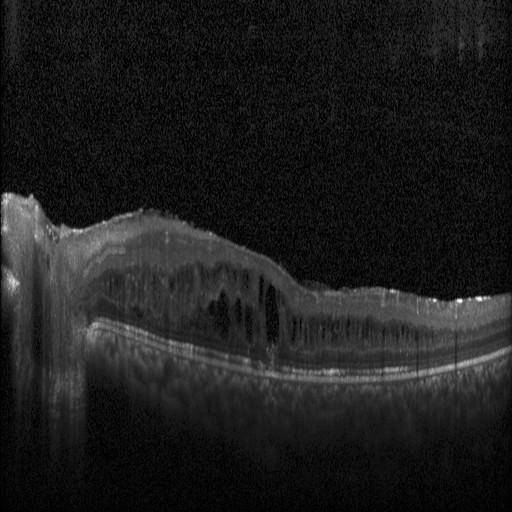
Retinal OCT cross-section.
Finding: DME.